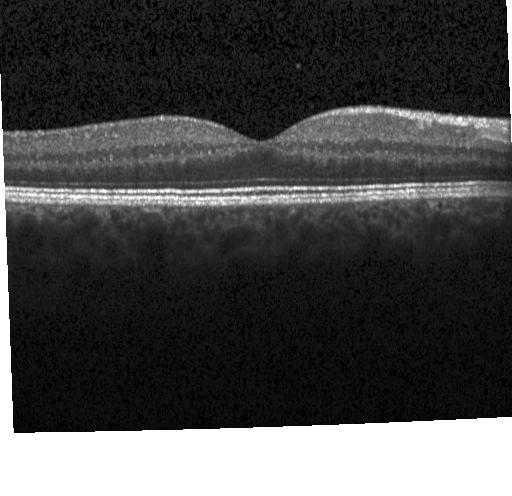 Horizontal scan through the fovea · OCT line scan · acquired on a Heidelberg Spectralis — This B-scan demonstrates no evidence of choroidal neovascularization, diabetic macular edema, or drusen.